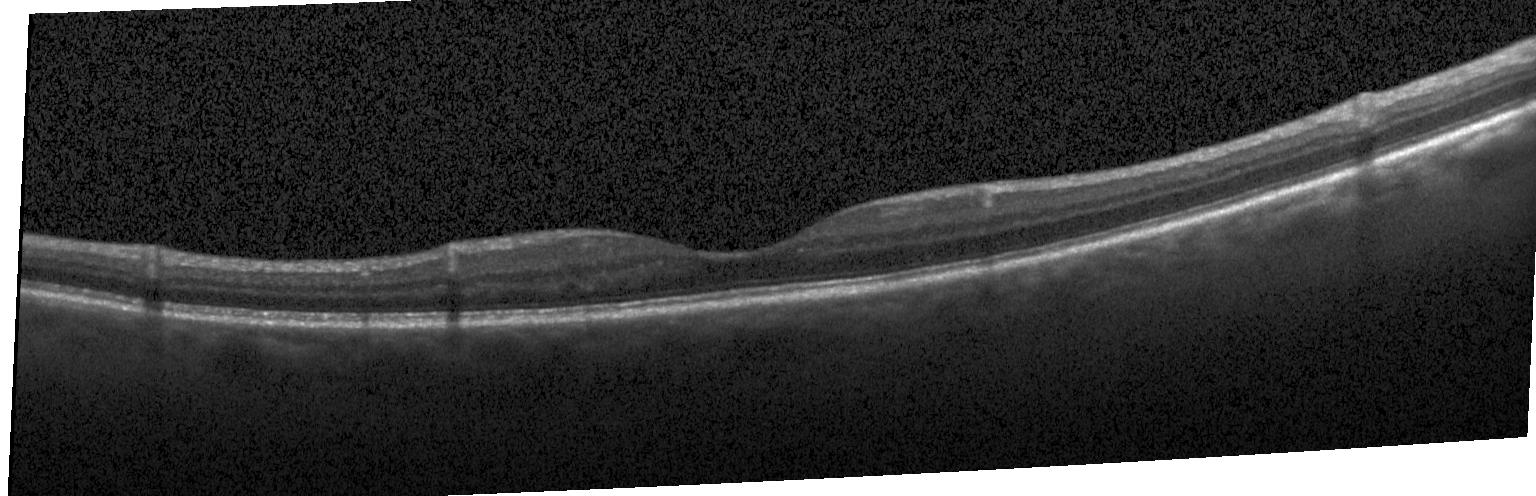
Macular scan. Optical coherence tomography scan.
Macular OCT: neither choroidal neovascularization, diabetic macular edema, nor drusen.